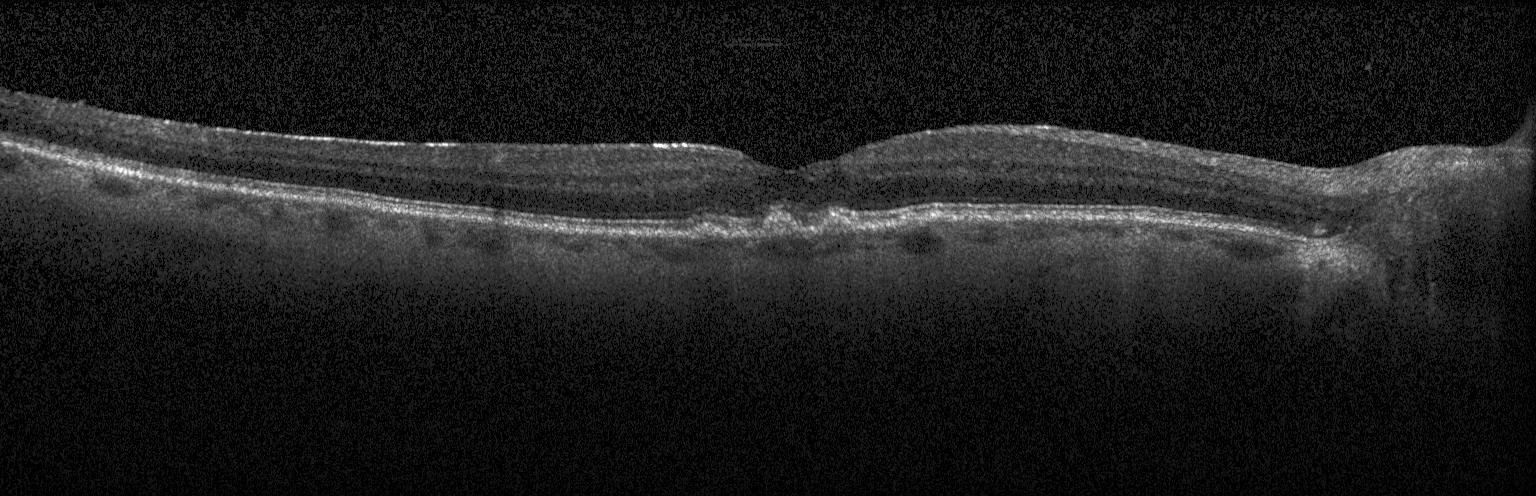 Through the macula · SD-OCT · optical coherence tomography B-scan · acquired on a Heidelberg Spectralis.
Assessment: multiple drusen.